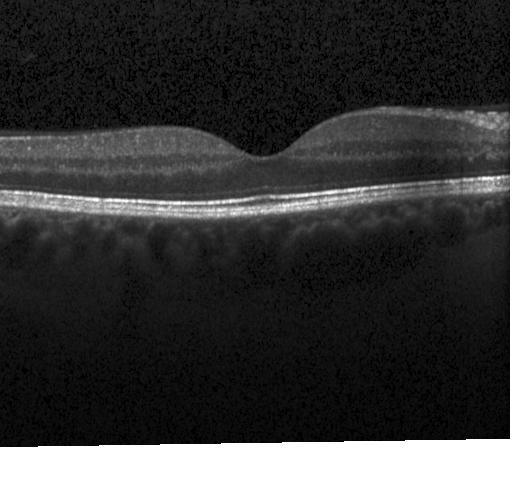

Spectral-domain OCT B-scan: no evidence of choroidal neovascularization, diabetic macular edema, or drusen.